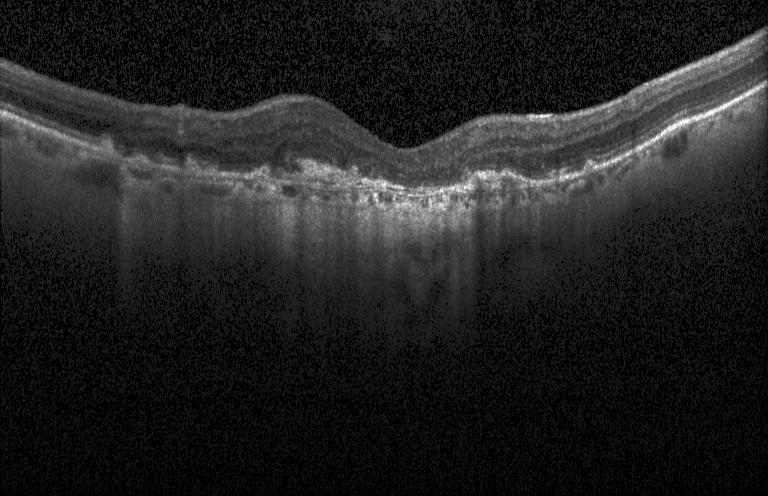
Macular scan. Spectral-domain optical coherence tomography. Optical coherence tomography B-scan. The scan shows choroidal neovascularization.